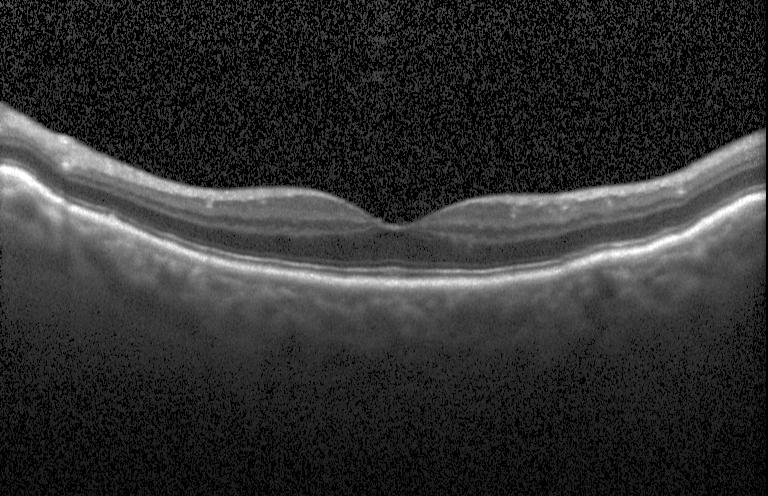
Horizontal scan through the fovea; retinal OCT B-scan — This B-scan demonstrates no choroidal neovascularization, no diabetic macular edema, and no drusen.